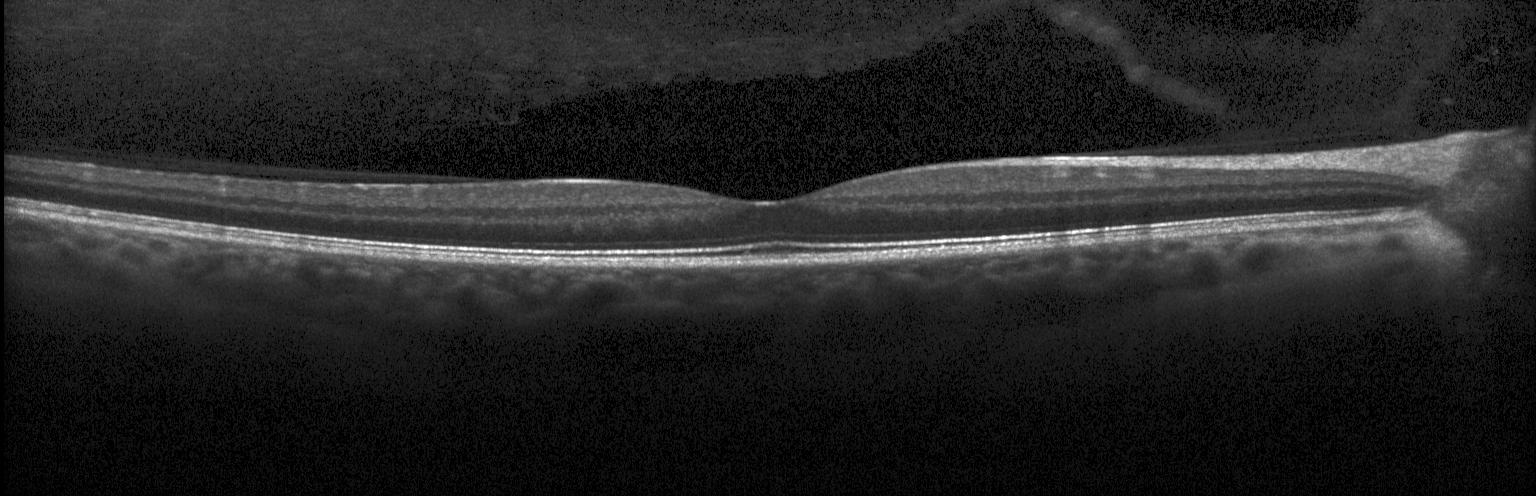

Optical coherence tomography scan
Macular OCT: no evidence of CNV, DME, or drusen.